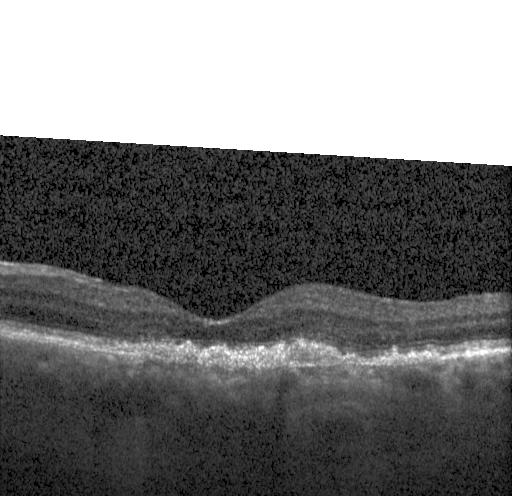
Retinal OCT B-scan. The scan shows choroidal neovascularization.